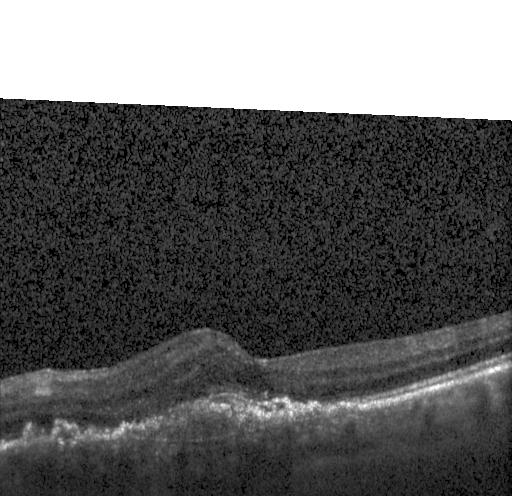 Diagnosis: a choroidal neovascular membrane.